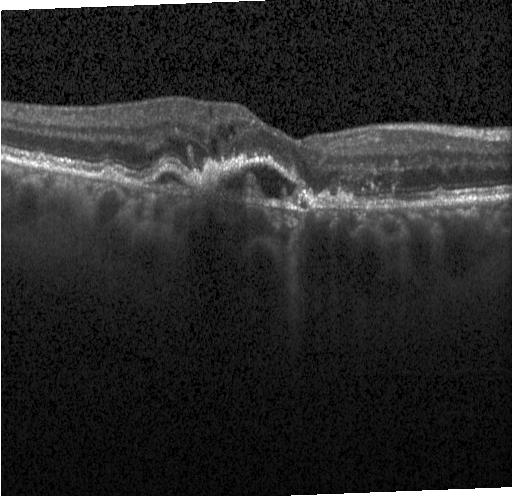
Fovea-centered, spectral-domain optical coherence tomography, acquired on a Heidelberg Spectralis, optical coherence tomography scan.
Dx: a choroidal neovascular membrane.